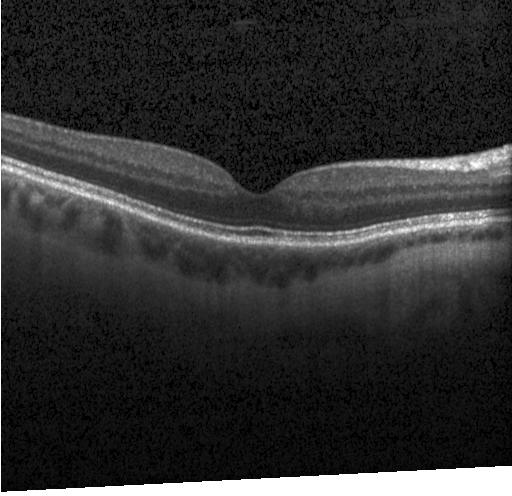 Retinal OCT cross-section · through the macula · instrument: Heidelberg Spectralis. This B-scan demonstrates neither choroidal neovascularization, diabetic macular edema, nor drusen.